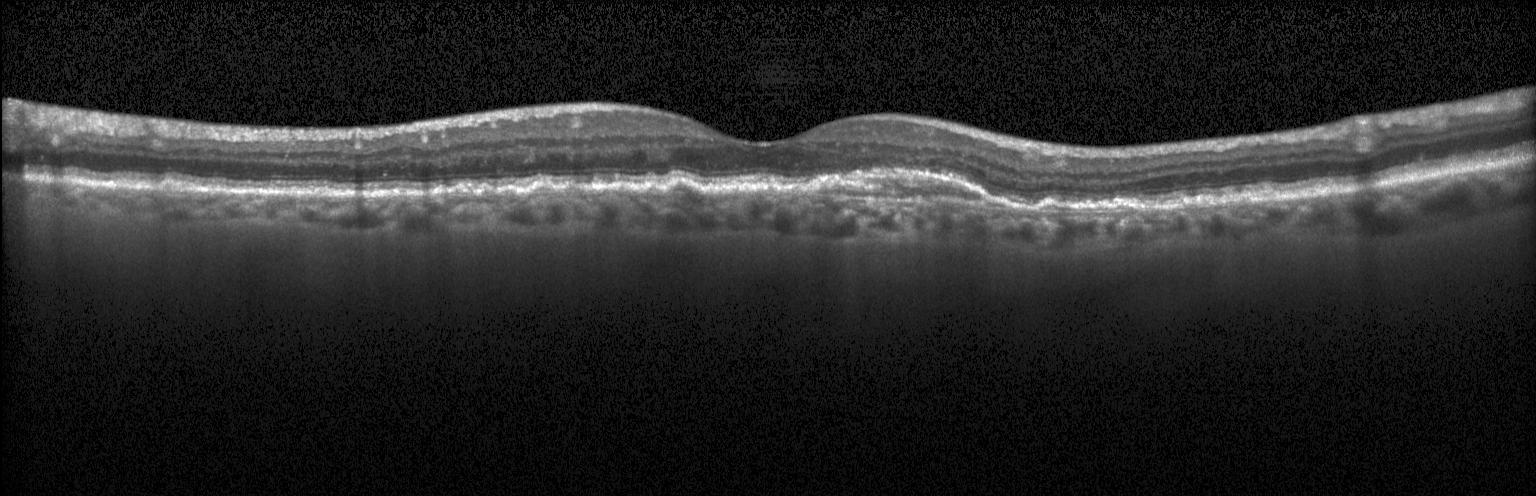 Impression: a choroidal neovascular membrane.